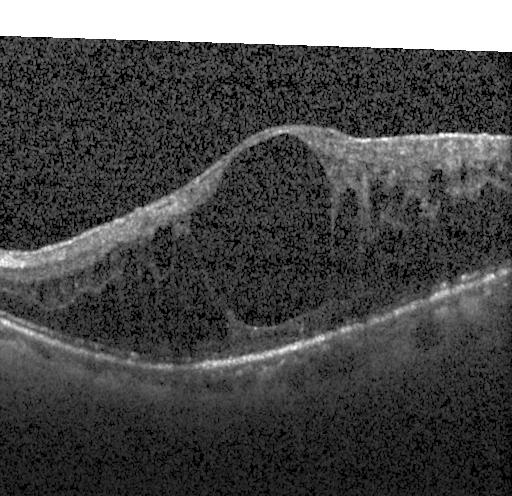
Retinal OCT cross-section
Finding: DME.